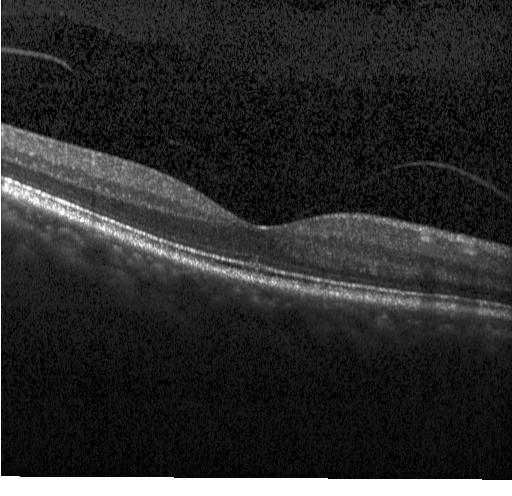

Diagnosis: no choroidal neovascularization, diabetic macular edema, or drusen.